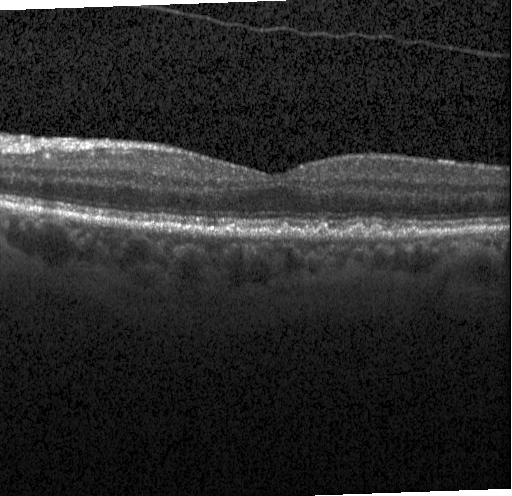

OCT B-scan — The scan shows drusen.